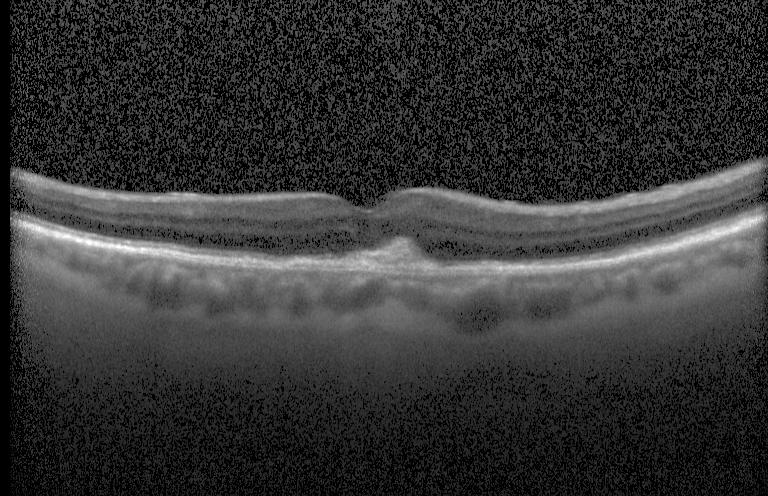

Macular OCT demonstrating choroidal neovascularization (CNV).